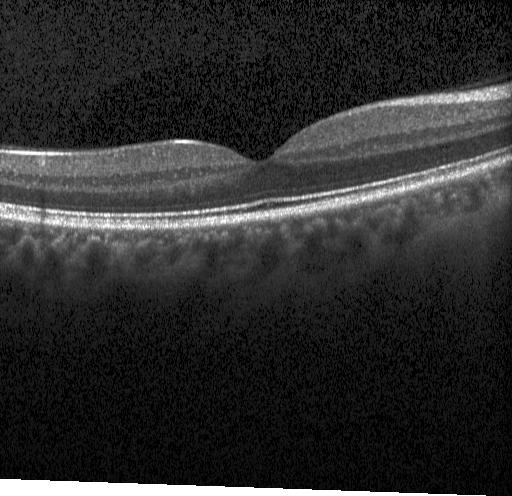
Instrument: Heidelberg Spectralis. SD-OCT. Retinal OCT cross-section. Macular scan — The scan shows neither choroidal neovascularization, diabetic macular edema, nor drusen.